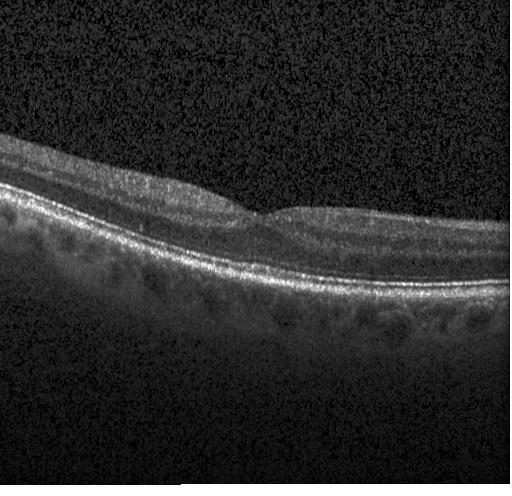 Instrument: Heidelberg Spectralis · SD-OCT · optical coherence tomography B-scan · fovea-centered
Impression: no evidence of choroidal neovascularization, diabetic macular edema, or drusen.